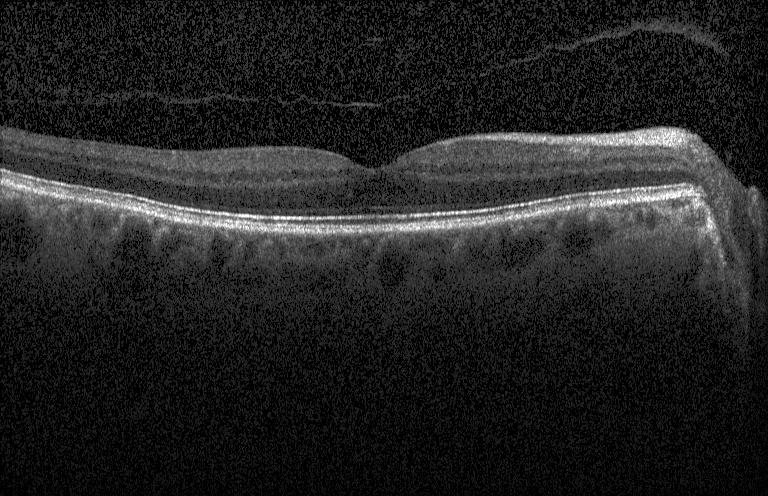
Retinal OCT cross-section showing no choroidal neovascularization, diabetic macular edema, or drusen.